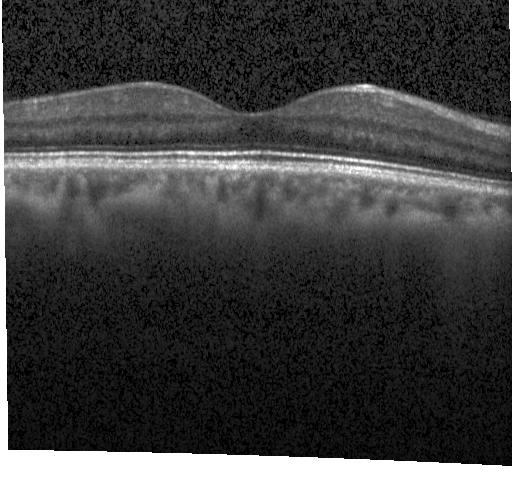

Heidelberg Spectralis OCT system. Optical coherence tomography B-scan. Diagnosis: no evidence of CNV, DME, or drusen.